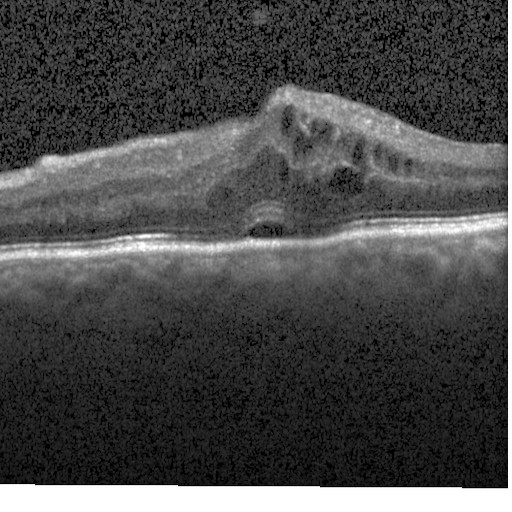
Retinal OCT B-scan, fovea-centered.
Impression: diabetic macular edema (DME).